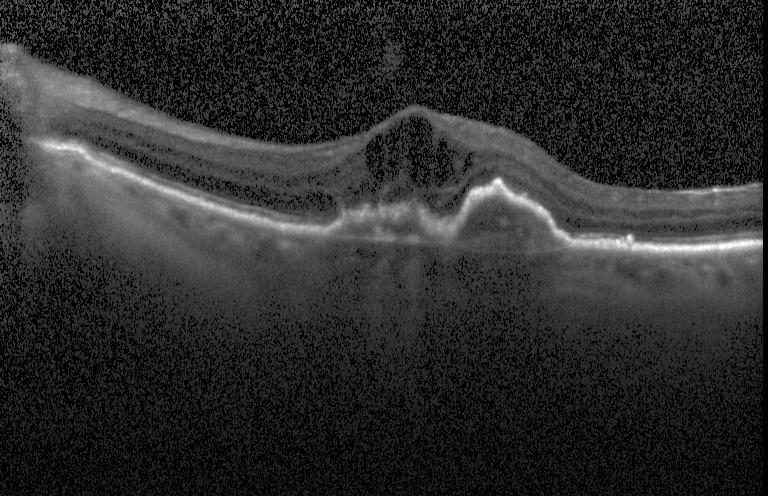

OCT B-scan showing a choroidal neovascular membrane.